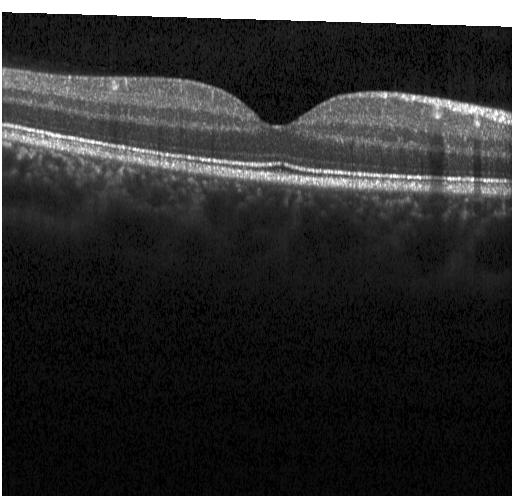 Dx: neither choroidal neovascularization, diabetic macular edema, nor drusen.